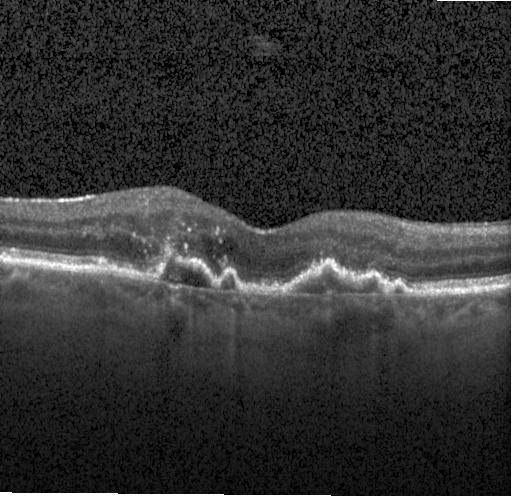

Through the macula, OCT B-scan.
Diagnosis: a choroidal neovascular membrane.